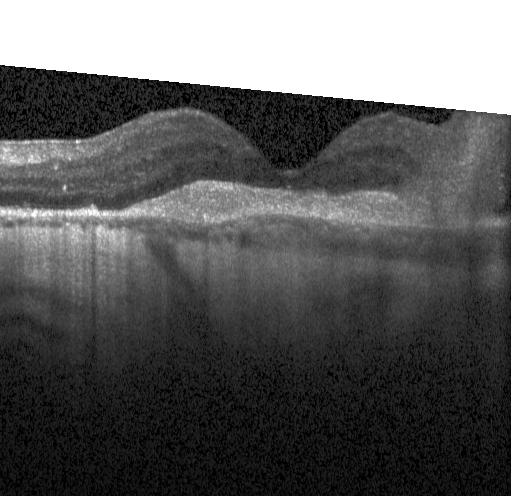
Horizontal scan through the fovea · OCT B-scan · spectral-domain OCT. Choroidal neovascularization (CNV).